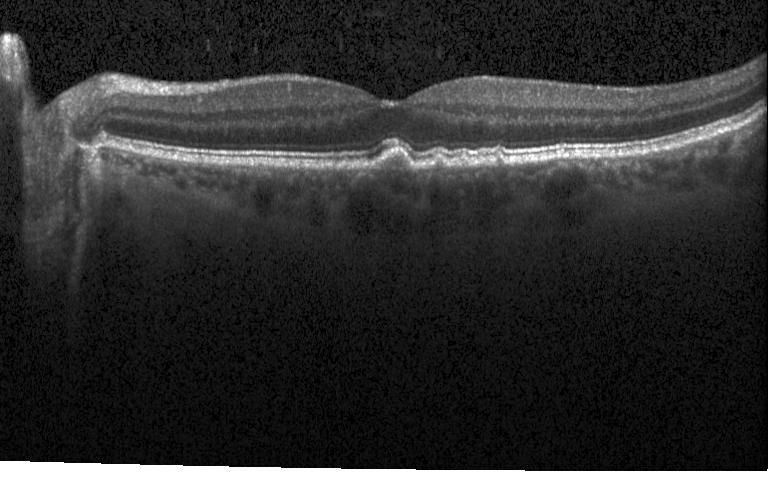
OCT scan showing drusen.